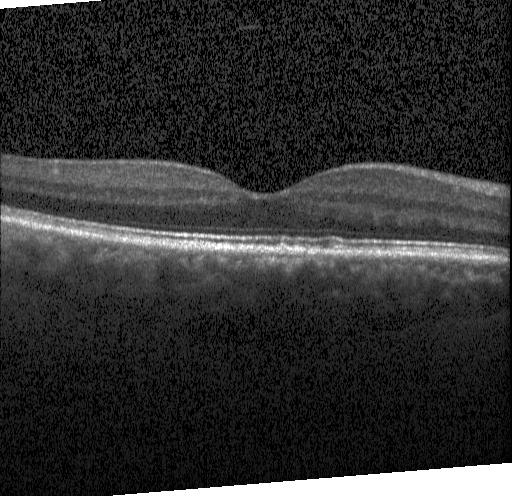 Optical coherence tomography scan. Instrument: Heidelberg Spectralis. Spectral-domain OCT. Through the macula
Finding: no choroidal neovascularization, diabetic macular edema, or drusen.